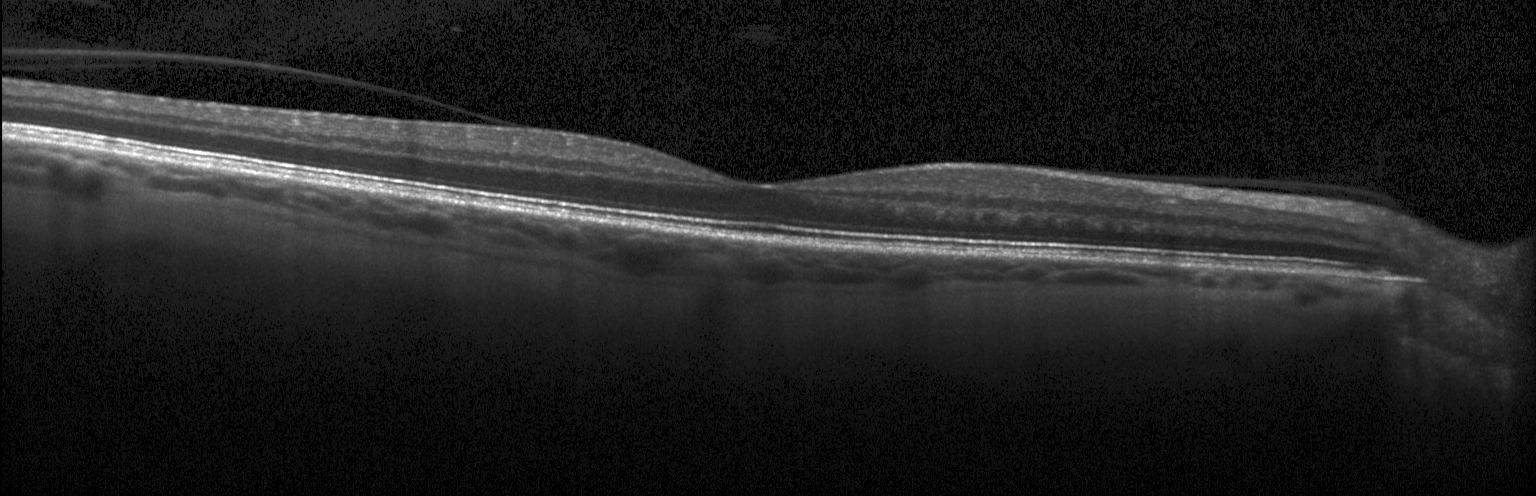 OCT line scan. Macular OCT: no evidence of CNV, DME, or drusen.